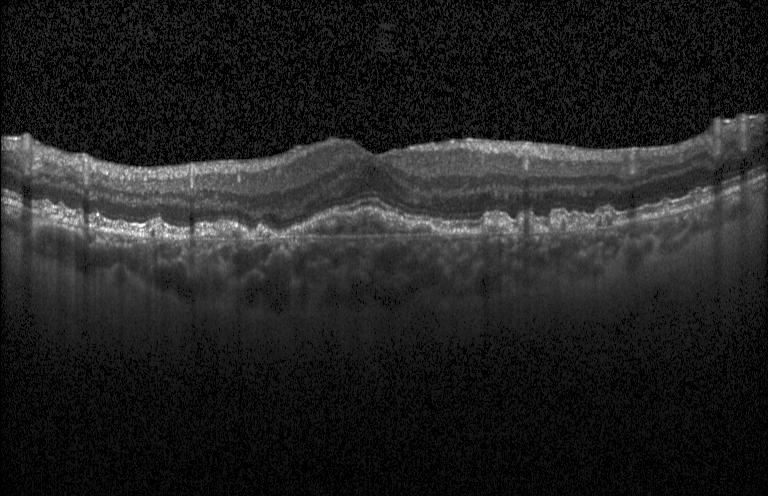 Impression: CNV.